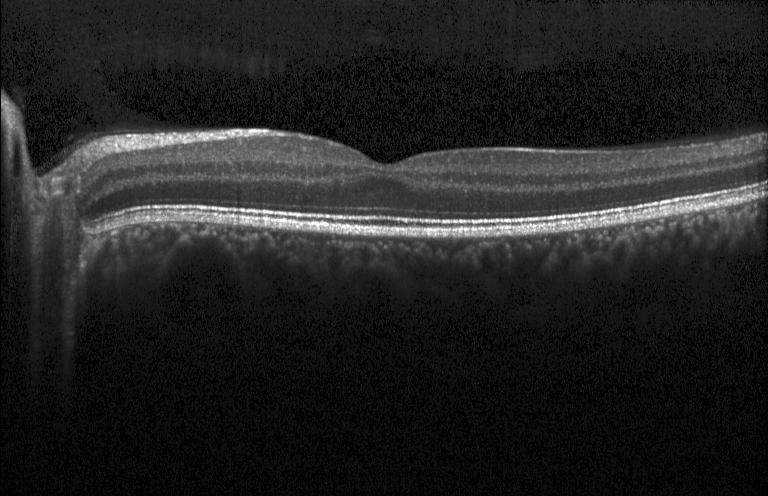 Diagnosis: no choroidal neovascularization, diabetic macular edema, or drusen.